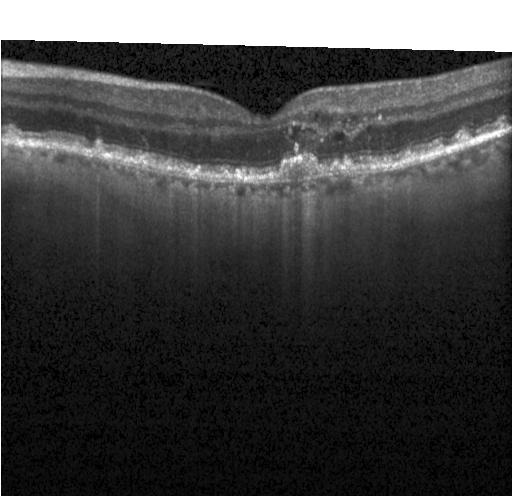 Optical coherence tomography scan.
This B-scan demonstrates CNV.